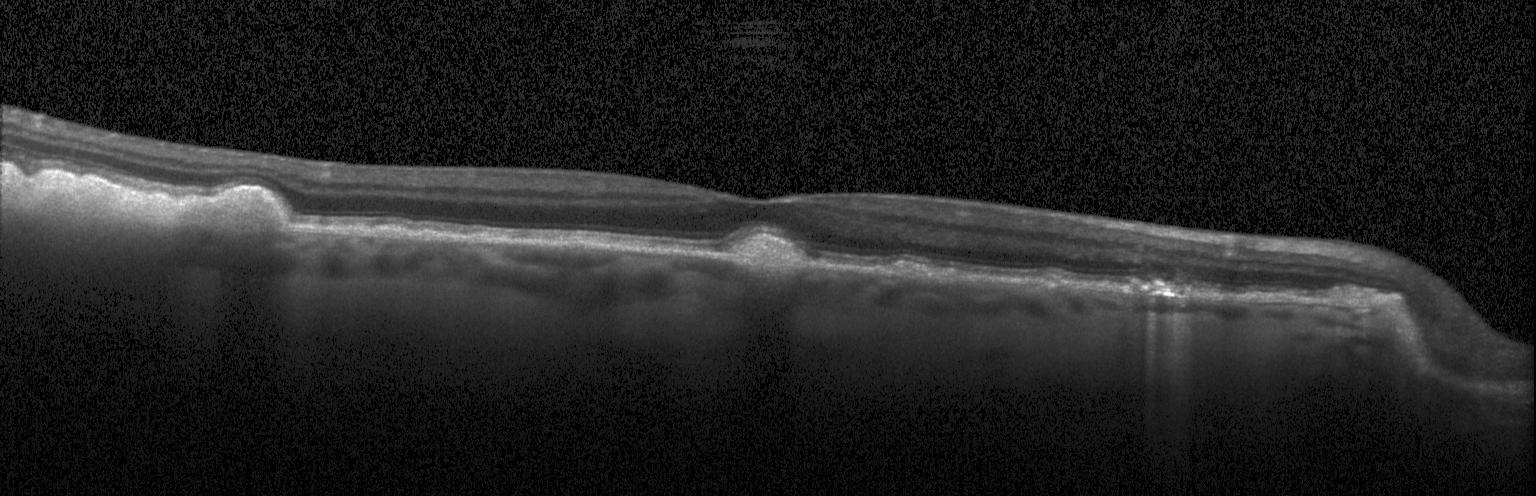

Instrument: Heidelberg Spectralis, optical coherence tomography B-scan, through the macula — Finding: drusen.